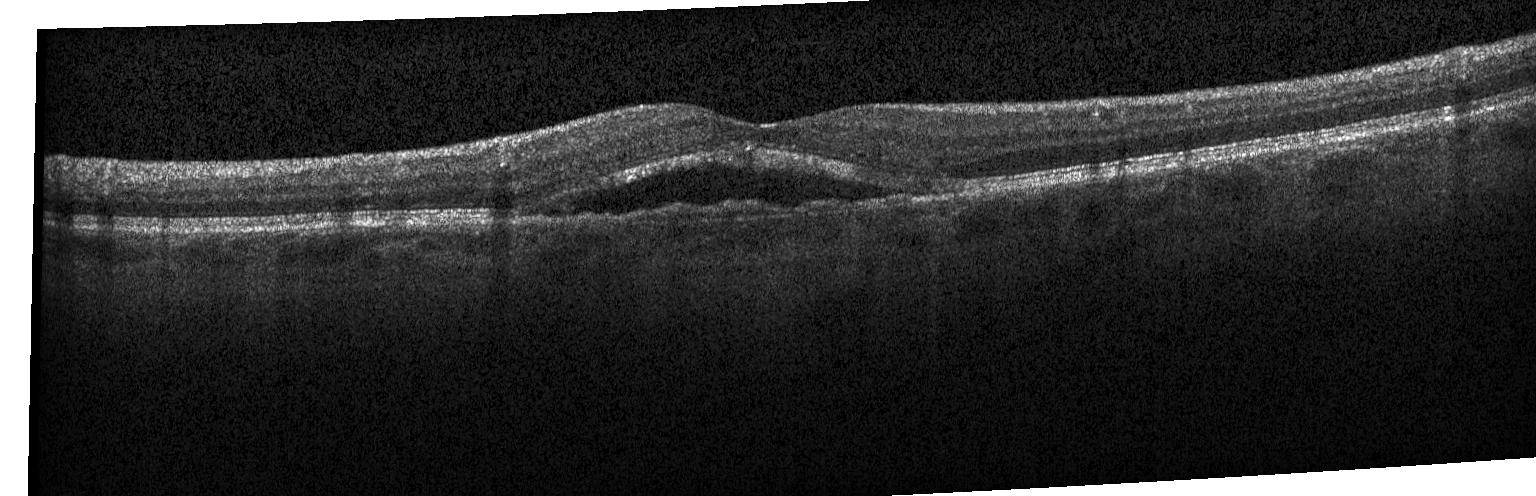

Macular scan · instrument: Heidelberg Spectralis · OCT B-scan · SD-OCT — Finding: choroidal neovascularization.